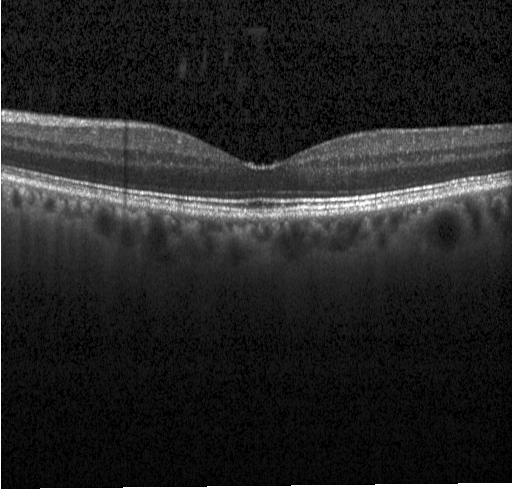

Fovea-centered, OCT line scan, spectral-domain optical coherence tomography, Heidelberg Spectralis OCT system. Finding: no evidence of choroidal neovascularization, diabetic macular edema, or drusen.